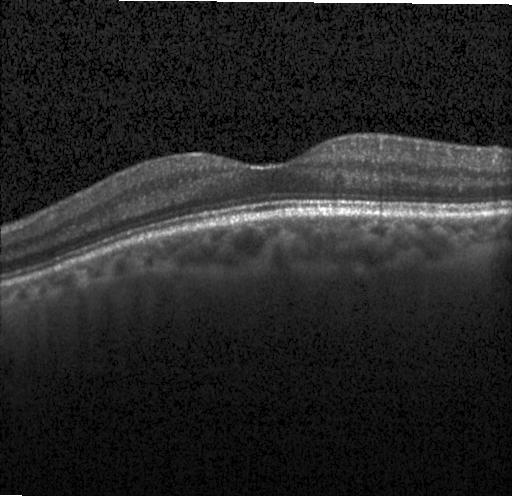
OCT line scan, acquired on a Heidelberg Spectralis
Macular OCT: no evidence of CNV, DME, or drusen.